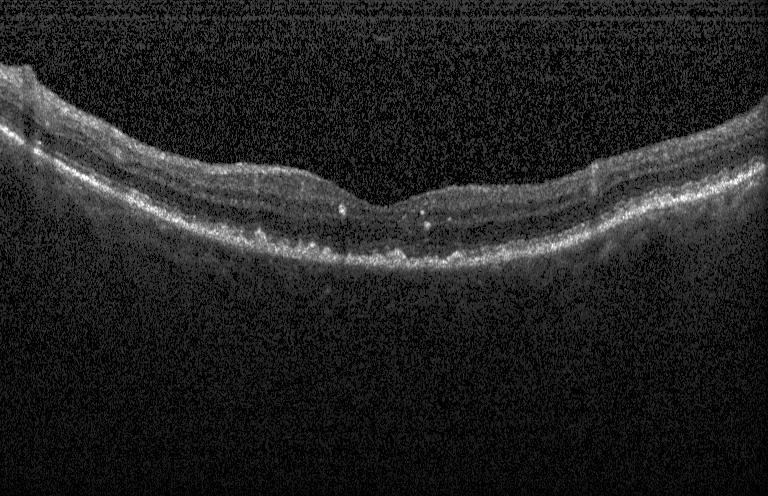

Optical coherence tomography scan. Macular scan. Heidelberg Spectralis
Impression: a choroidal neovascular membrane.